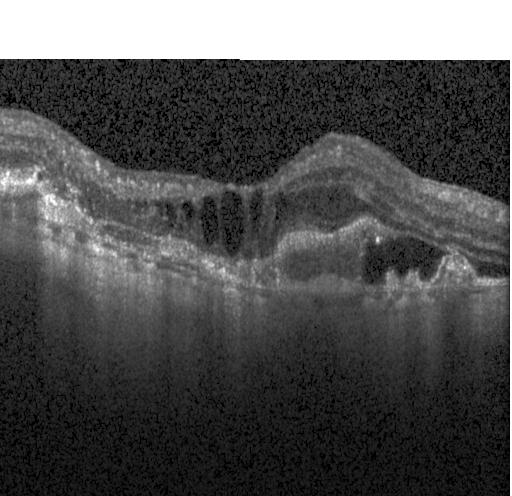 OCT finding: a choroidal neovascular membrane.